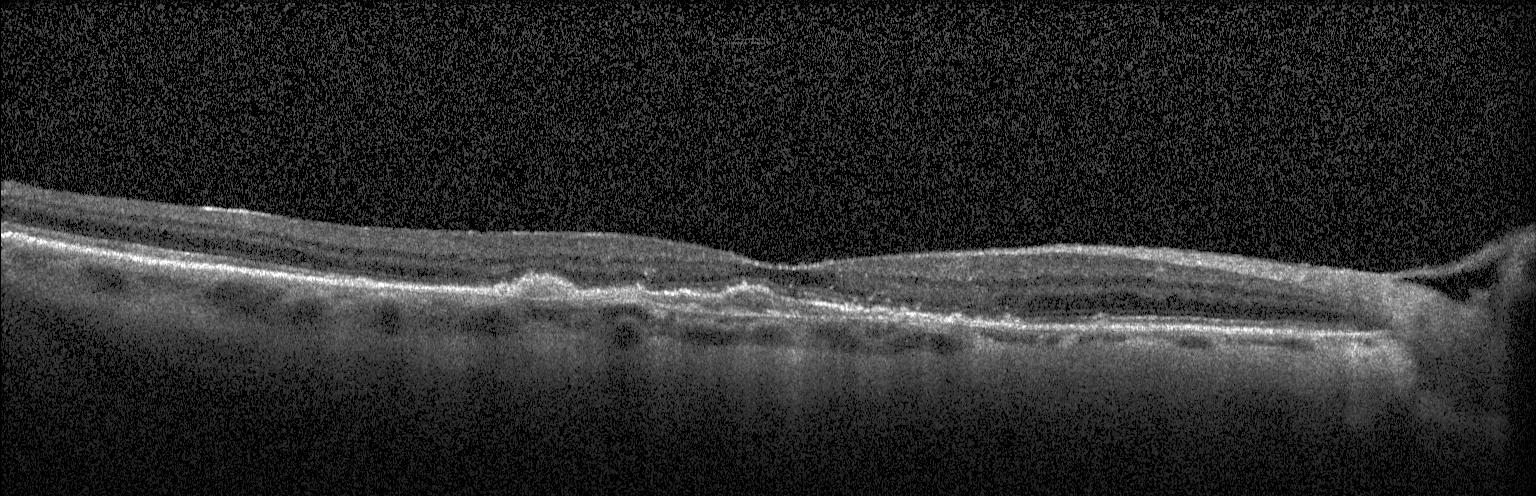 Assessment: choroidal neovascularization.